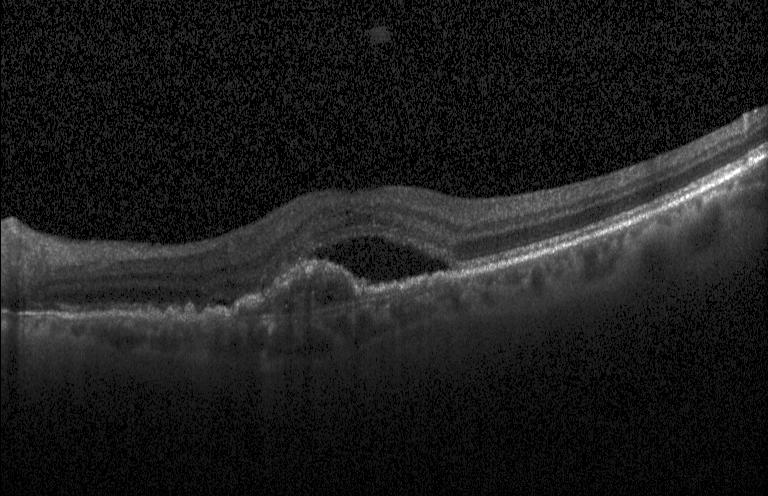 The scan shows a choroidal neovascular membrane.